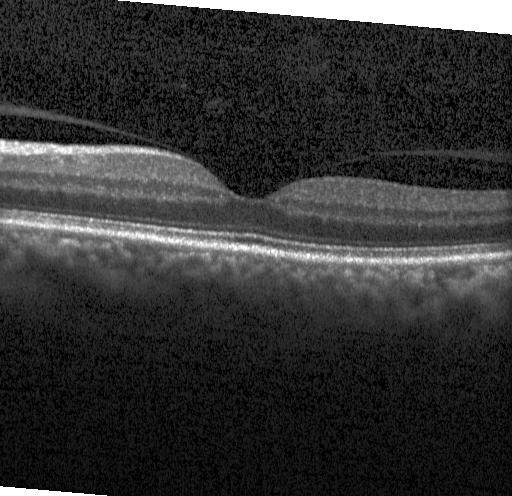

OCT finding: neither choroidal neovascularization, diabetic macular edema, nor drusen.